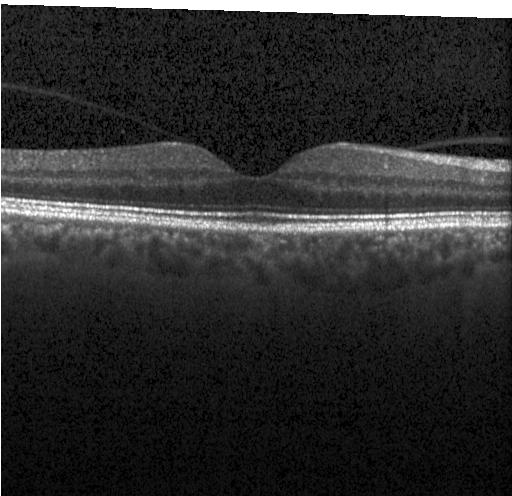 Assessment: no choroidal neovascularization, diabetic macular edema, or drusen.